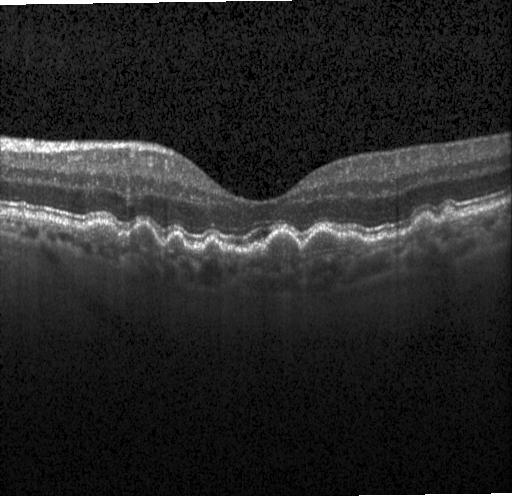 The scan shows drusen.